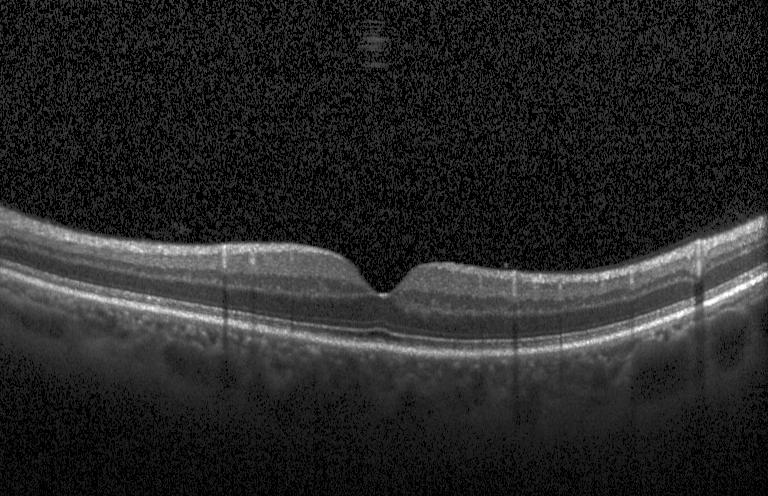 OCT B-scan showing no CNV, no DME, and no drusen.